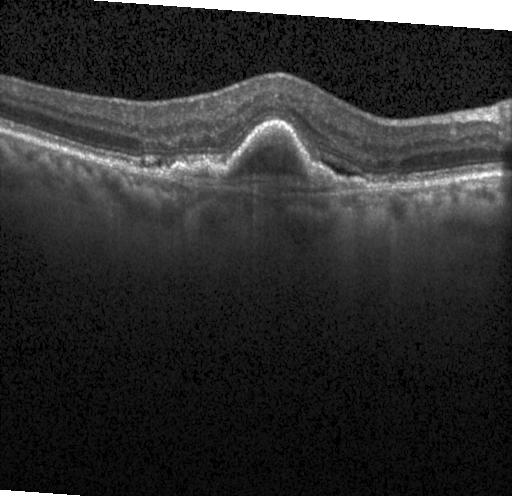
OCT B-scan
This B-scan demonstrates a choroidal neovascular membrane.